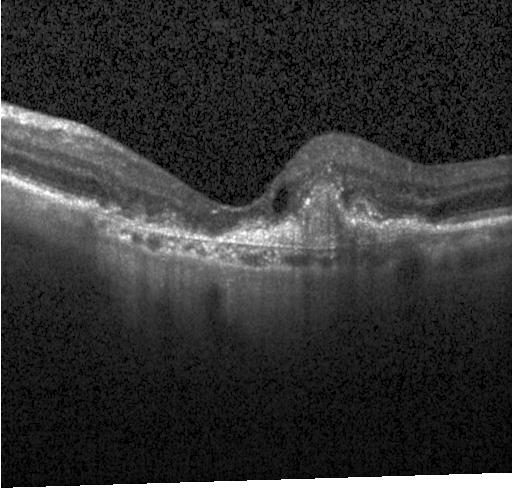
OCT B-scan showing choroidal neovascularization.